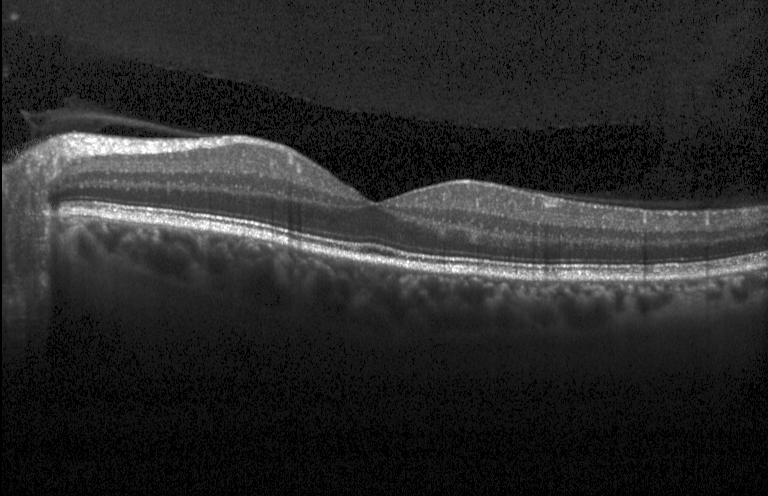
Macular OCT demonstrating neither choroidal neovascularization, diabetic macular edema, nor drusen.